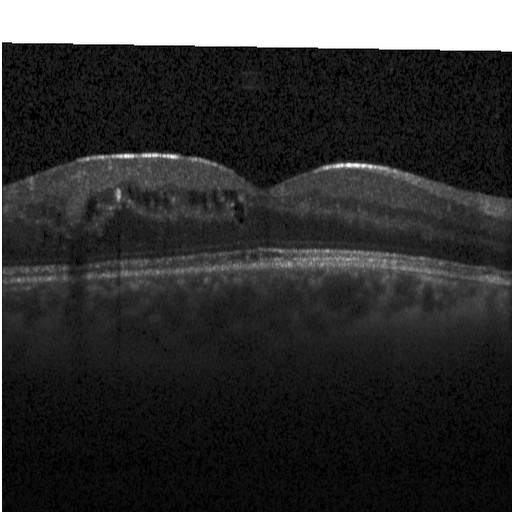
Impression: diabetic macular edema.